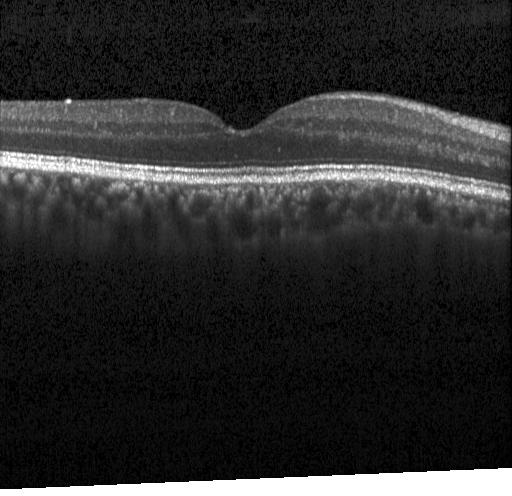
Macular OCT: no evidence of CNV, DME, or drusen.